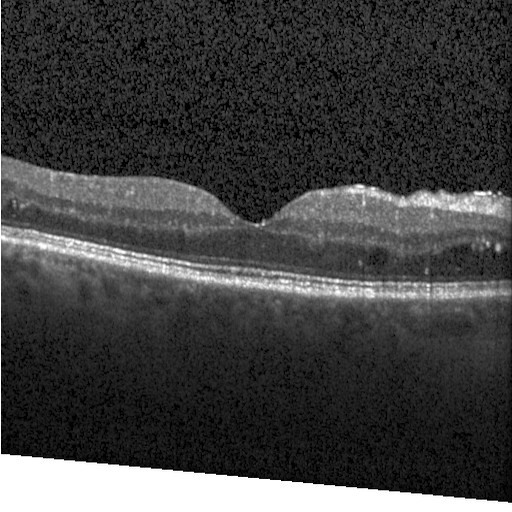

Impression: diabetic macular edema (DME).